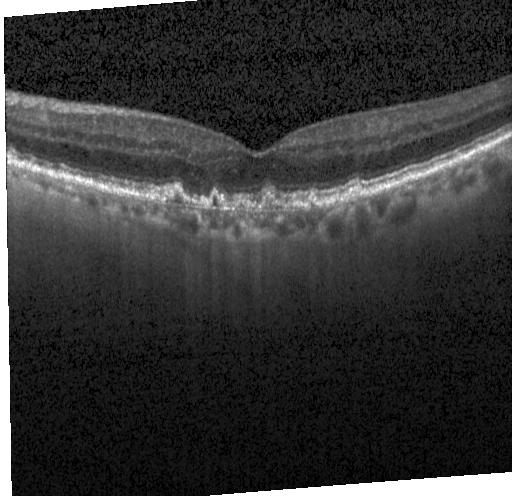
Horizontal scan through the fovea; Heidelberg Spectralis OCT system; retinal OCT cross-section; spectral-domain optical coherence tomography. OCT finding: multiple drusen.